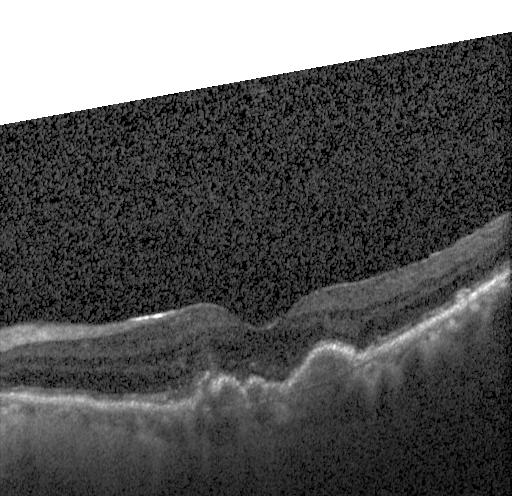

Macular scan, OCT B-scan.
OCT finding: a choroidal neovascular membrane.